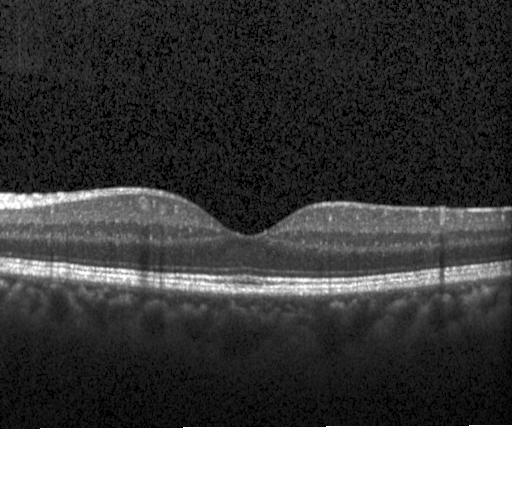 Spectral-domain OCT · centered on the fovea · optical coherence tomography B-scan · instrument: Heidelberg Spectralis. Impression: no choroidal neovascularization, no diabetic macular edema, and no drusen.